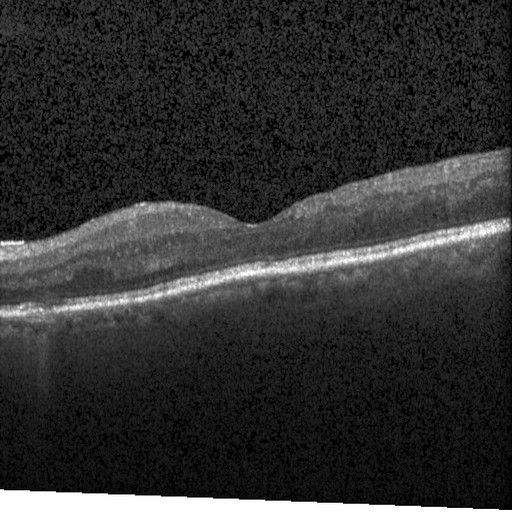
OCT B-scan showing diabetic macular edema.